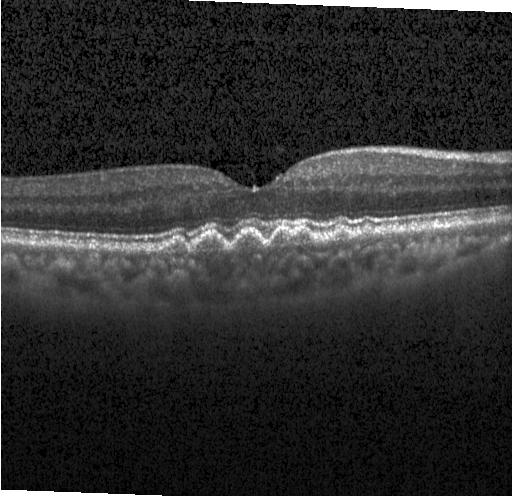

Optical coherence tomography B-scan; fovea-centered; instrument: Heidelberg Spectralis; spectral-domain optical coherence tomography — Sub-RPE drusenoid deposits.